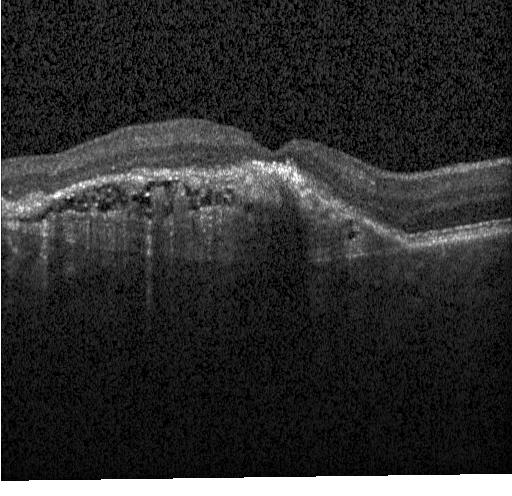

Spectral-domain optical coherence tomography · optical coherence tomography scan
Macular OCT: CNV.